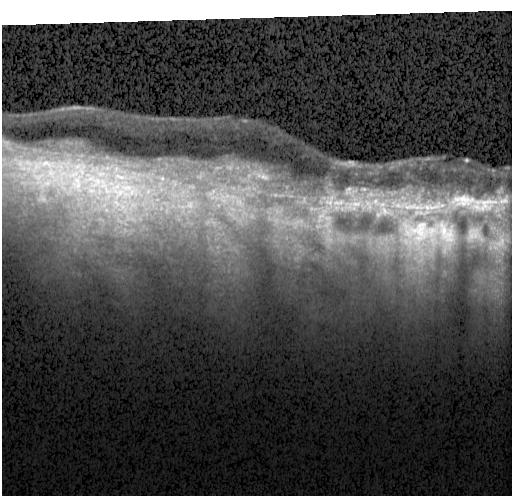
OCT B-scan — This B-scan demonstrates CNV.